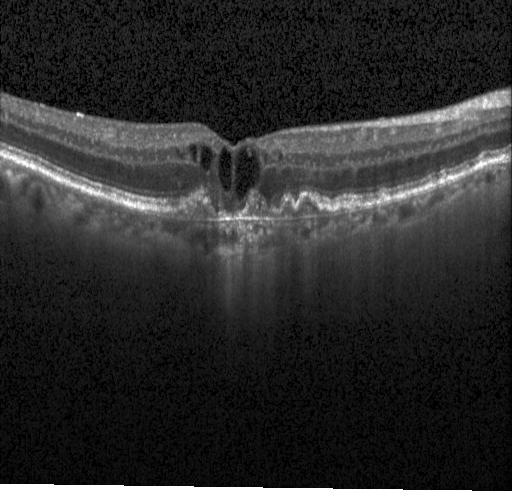

Fovea-centered · Heidelberg Spectralis OCT system · optical coherence tomography B-scan. Impression: CNV.